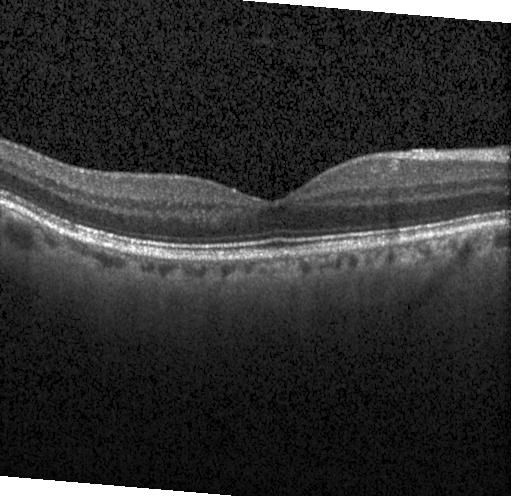 Optical coherence tomography B-scan. Impression: no evidence of choroidal neovascularization, diabetic macular edema, or drusen.